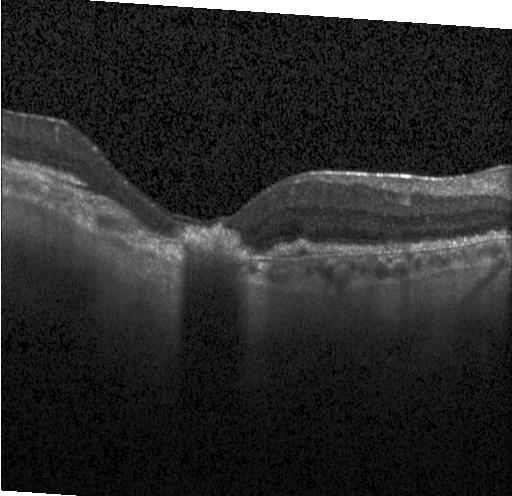
OCT scan showing CNV.